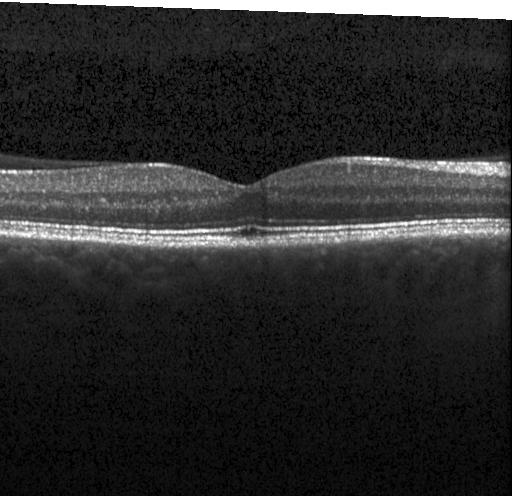

Retinal OCT cross-section.
Neither choroidal neovascularization, diabetic macular edema, nor drusen.